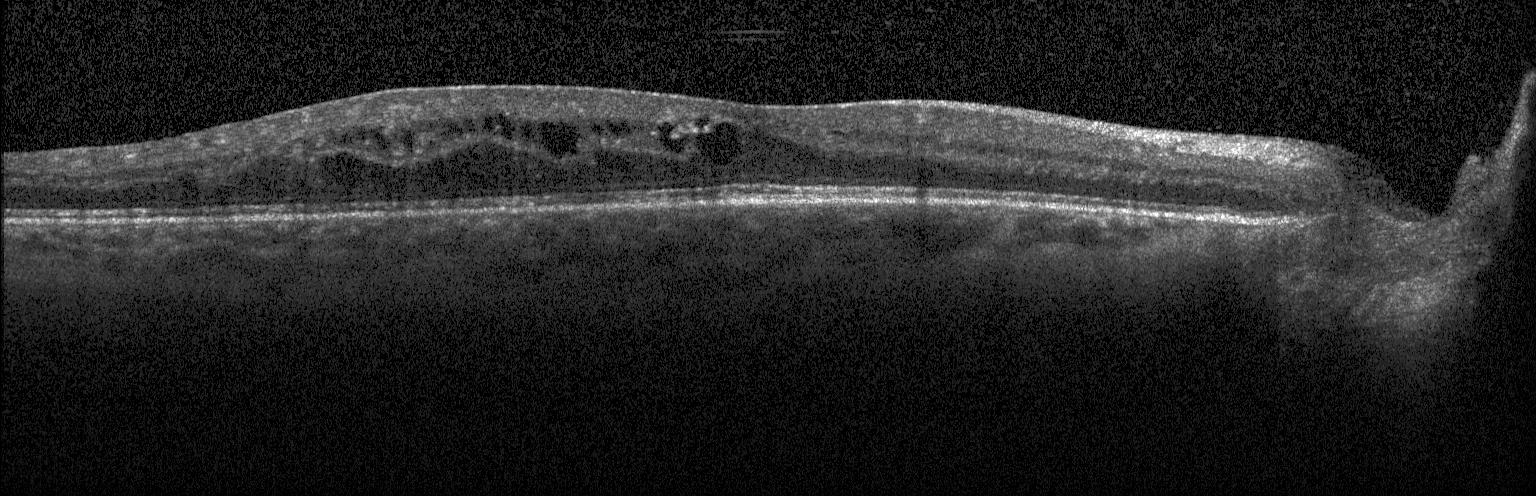
OCT B-scan · Heidelberg Spectralis · horizontal scan through the fovea — Dx: diabetic macular edema (DME).